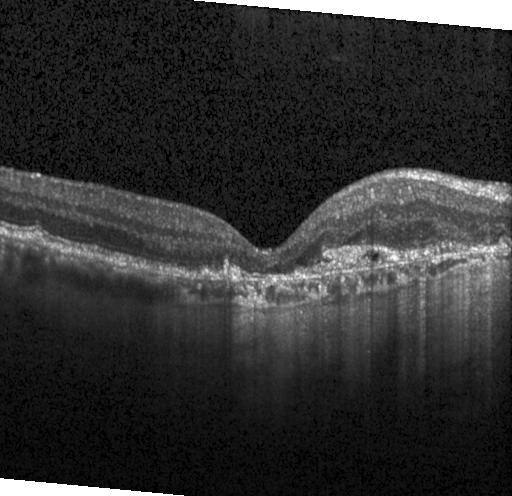

Diagnosis: choroidal neovascularization (CNV).